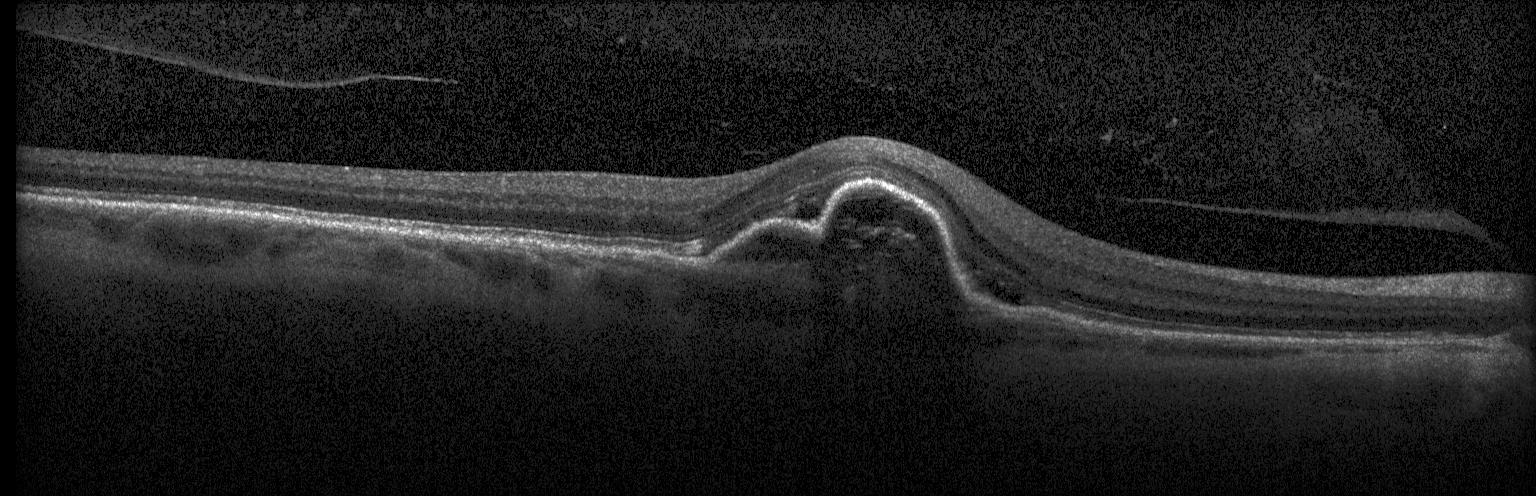

OCT B-scan.
Impression: a choroidal neovascular membrane.